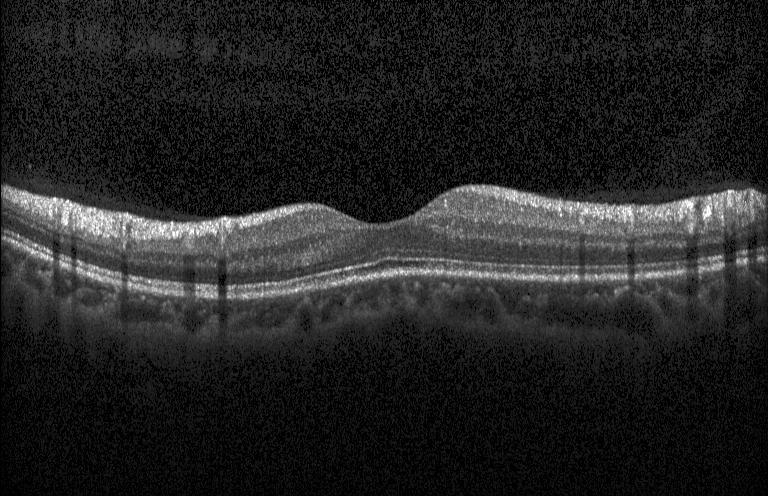
SD-OCT · retinal OCT B-scan. OCT finding: no choroidal neovascularization, diabetic macular edema, or drusen.